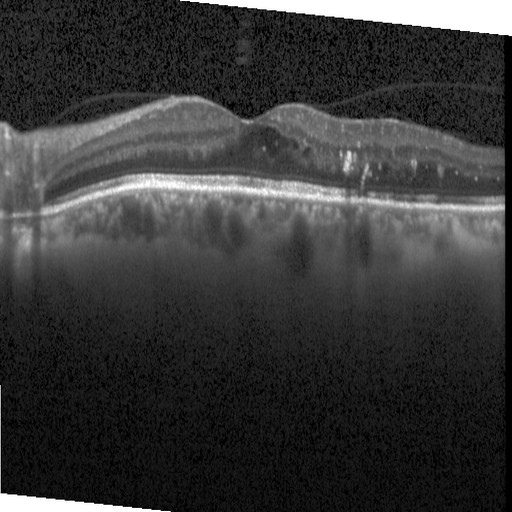 Retinal OCT cross-section · through the macula · SD-OCT · instrument: Heidelberg Spectralis.
Finding: diabetic macular edema (DME).